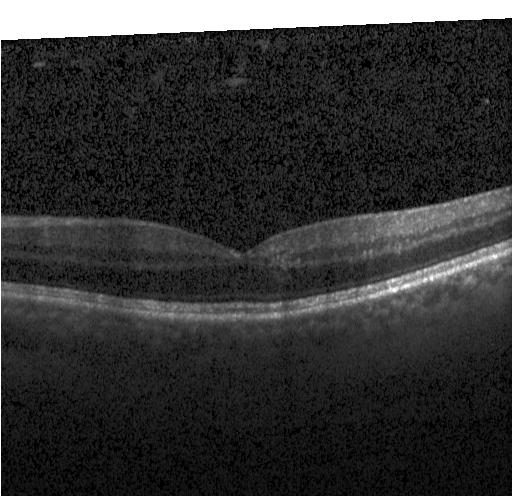 Spectral-domain optical coherence tomography, centered on the fovea, acquired on a Heidelberg Spectralis, retinal OCT cross-section — Finding: no CNV, DME, or drusen.